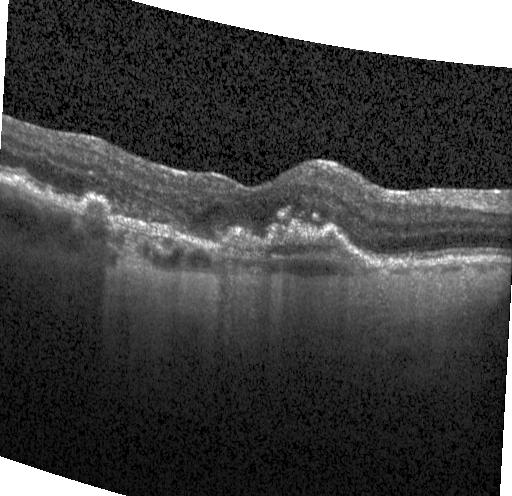

OCT B-scan — Finding: a choroidal neovascular membrane.